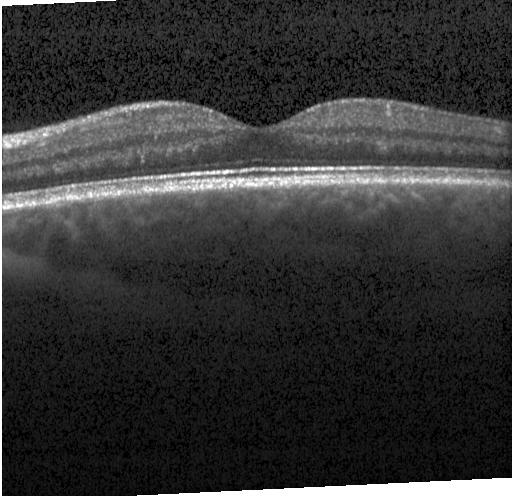
The scan shows no CNV, no DME, and no drusen.